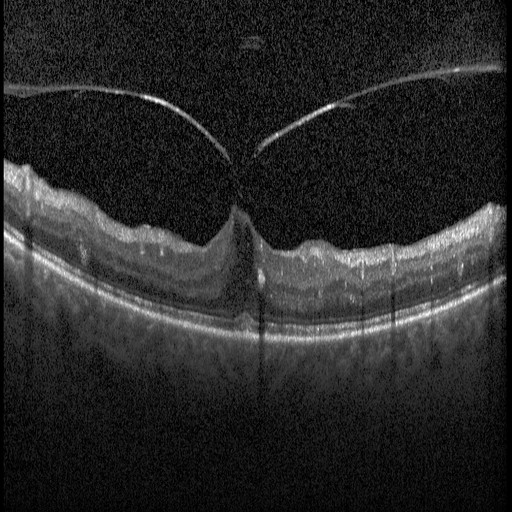 Diagnosis: diabetic macular edema (DME).